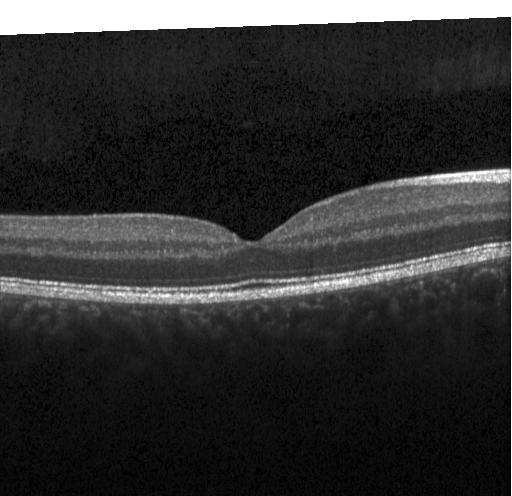 Optical coherence tomography scan.
Finding: no CNV, DME, or drusen.